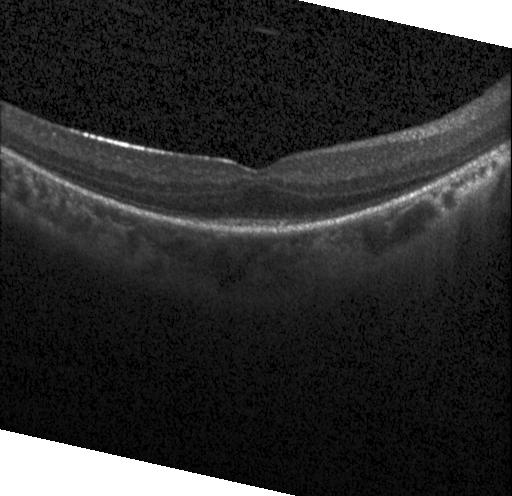 Macular OCT demonstrating neither choroidal neovascularization, diabetic macular edema, nor drusen.